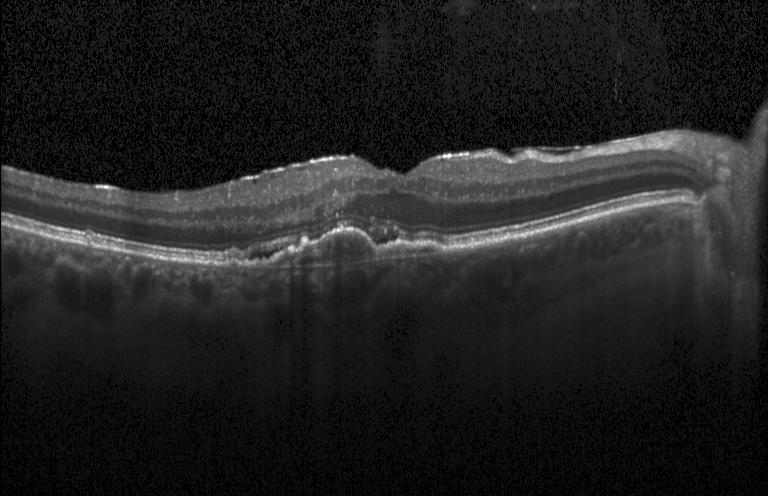
OCT scan showing a choroidal neovascular membrane.